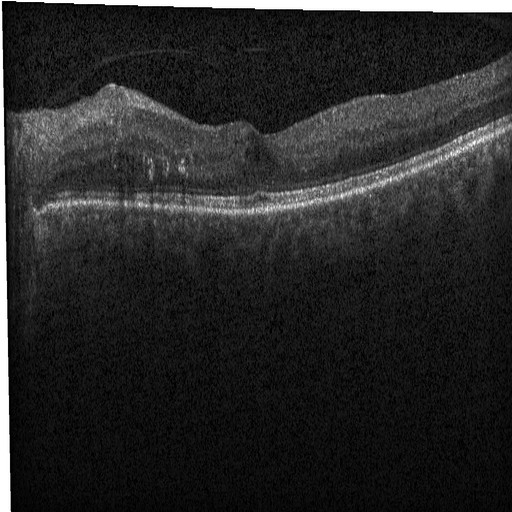

Retinal OCT cross-section, Heidelberg Spectralis — Finding: DME.